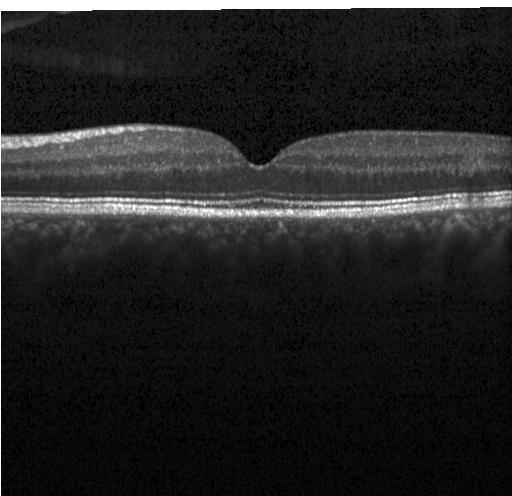
Macular OCT: no evidence of CNV, DME, or drusen.